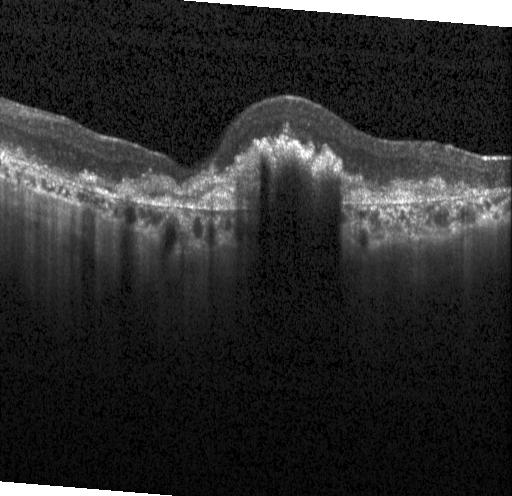 A choroidal neovascular membrane.